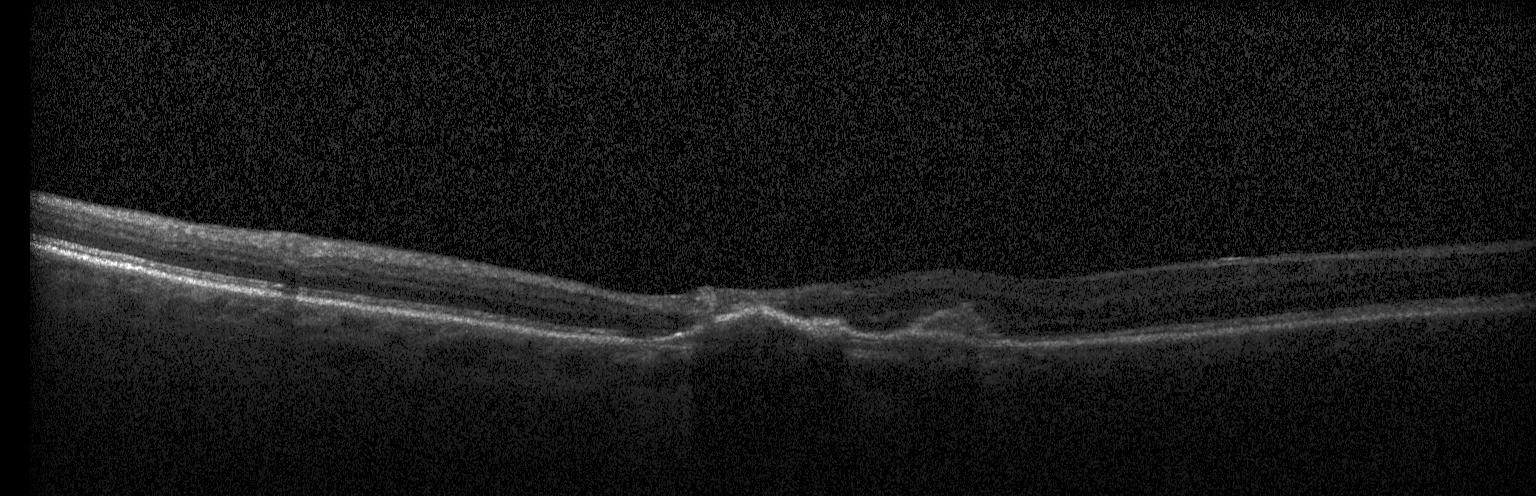
Spectral-domain OCT · acquired on a Heidelberg Spectralis · OCT line scan.
Dx: a choroidal neovascular membrane.